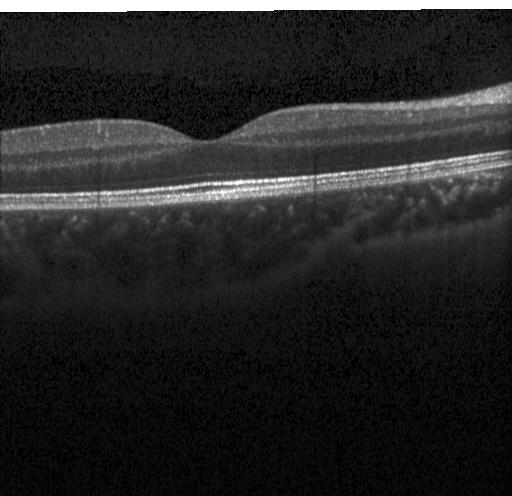 SD-OCT · OCT line scan.
No evidence of choroidal neovascularization, diabetic macular edema, or drusen.